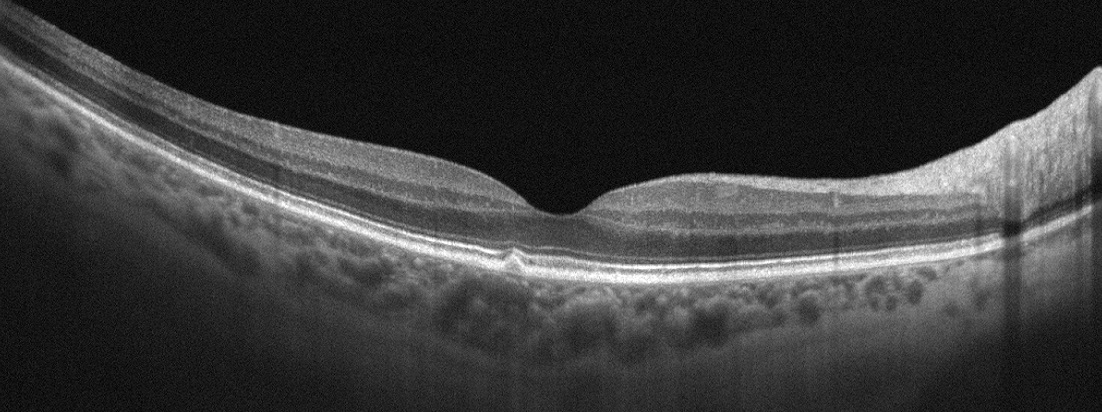
Macular OCT: age-related macular degeneration.